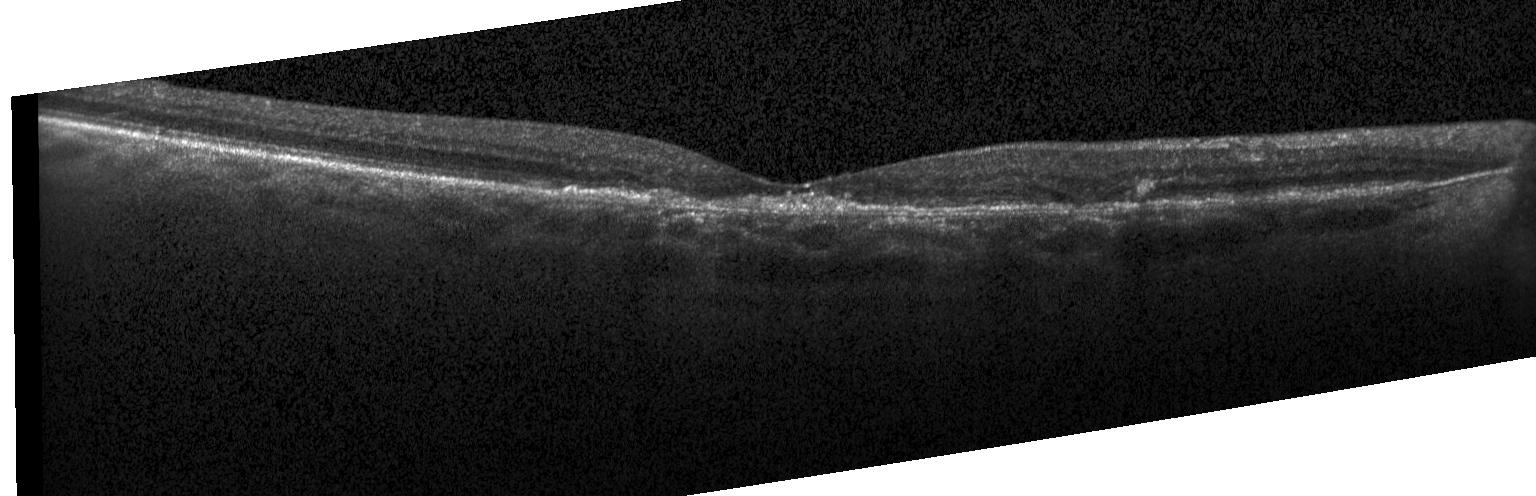 SD-OCT, retinal OCT B-scan.
Dx: a choroidal neovascular membrane.